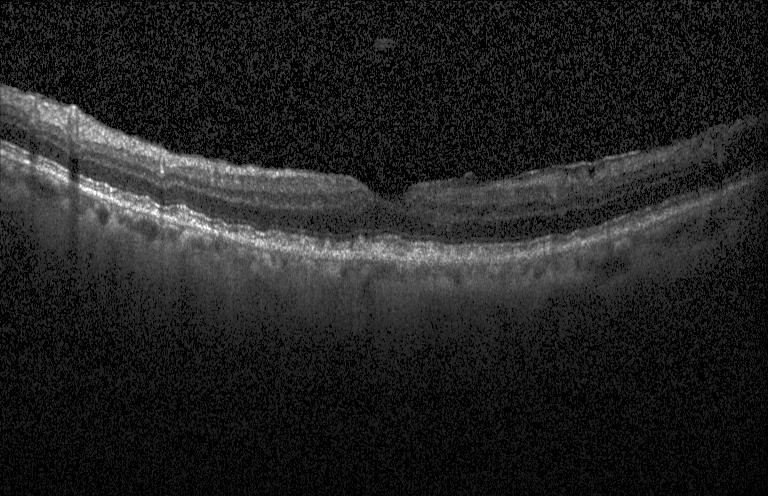
Centered on the fovea · Heidelberg Spectralis OCT system · OCT line scan · SD-OCT — Finding: drusen.